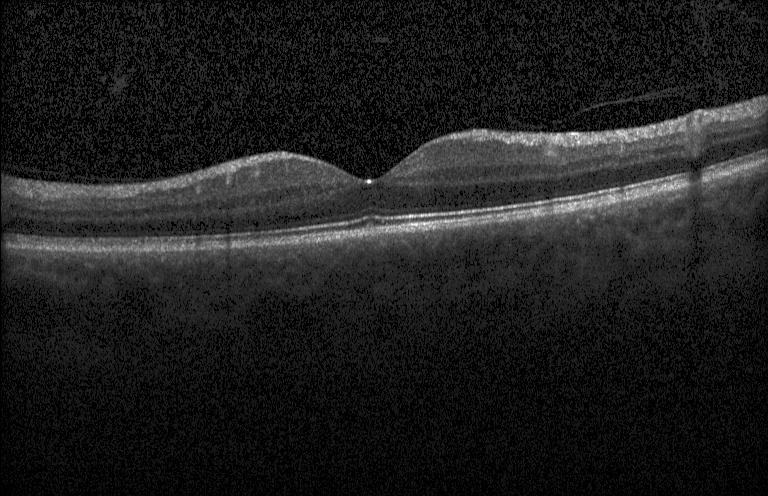

OCT line scan. Diagnosis: neither choroidal neovascularization, diabetic macular edema, nor drusen.